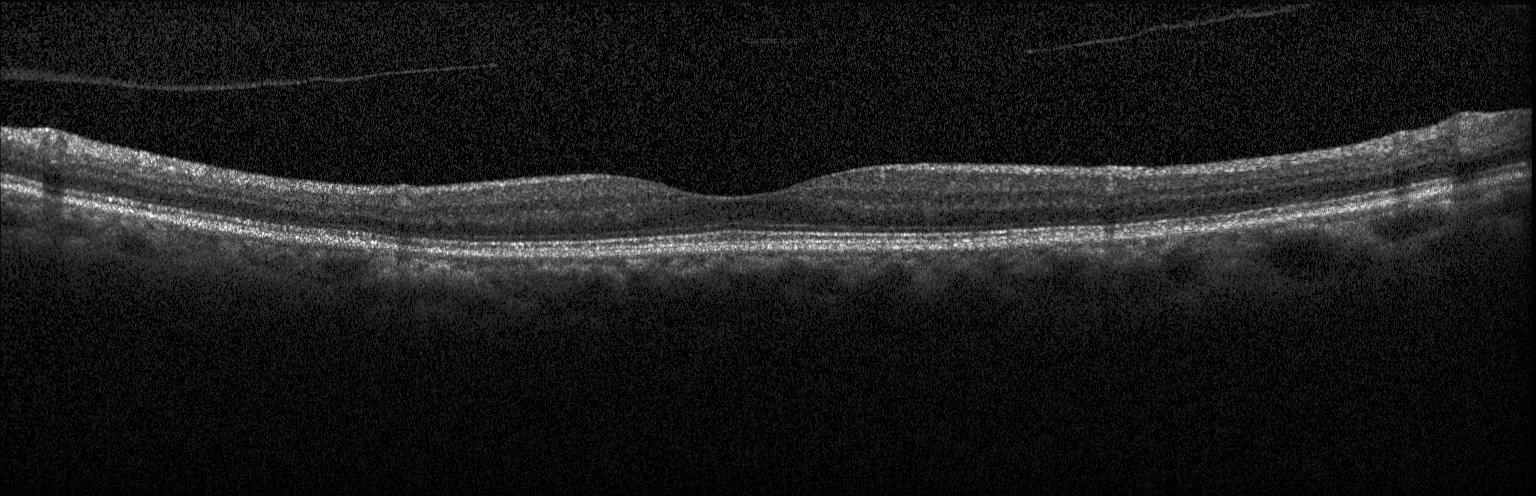 Spectral-domain OCT · centered on the fovea · optical coherence tomography B-scan
Dx: no evidence of CNV, DME, or drusen.